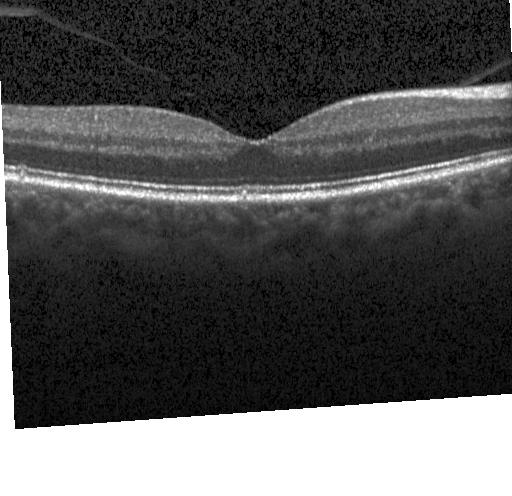

Spectral-domain OCT B-scan: neither choroidal neovascularization, diabetic macular edema, nor drusen.